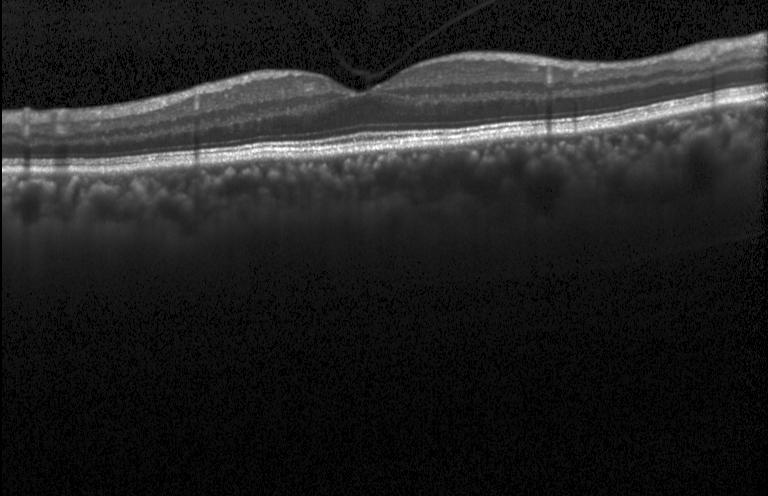

Heidelberg Spectralis · fovea-centered · OCT B-scan · SD-OCT
No choroidal neovascularization, diabetic macular edema, or drusen.